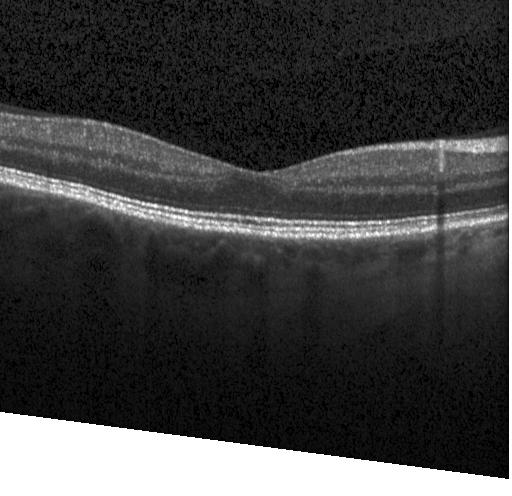
OCT line scan. Spectral-domain optical coherence tomography. Horizontal scan through the fovea.
OCT finding: neither CNV, DME, nor drusen.